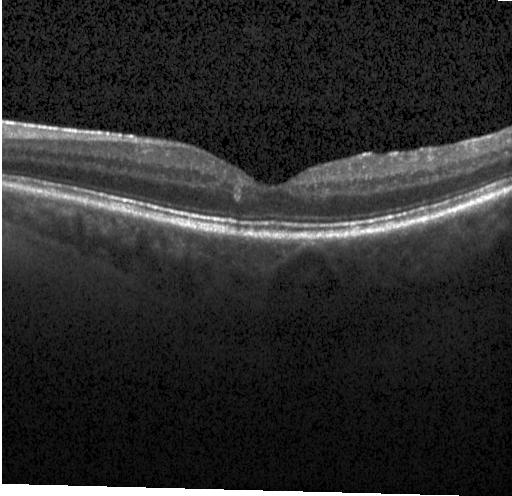

OCT finding: no evidence of CNV, DME, or drusen.